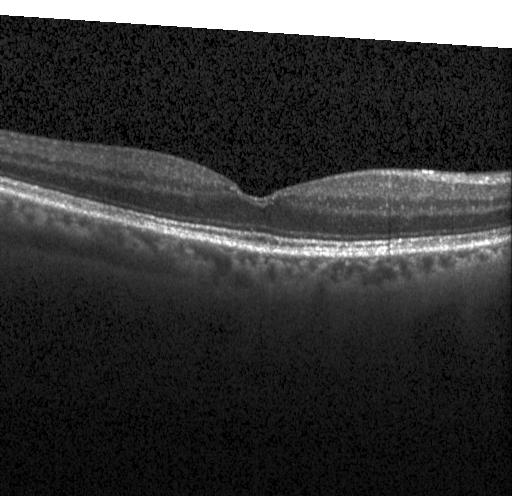

Spectral-domain optical coherence tomography, centered on the fovea, retinal OCT cross-section, Heidelberg Spectralis.
Finding: neither choroidal neovascularization, diabetic macular edema, nor drusen.